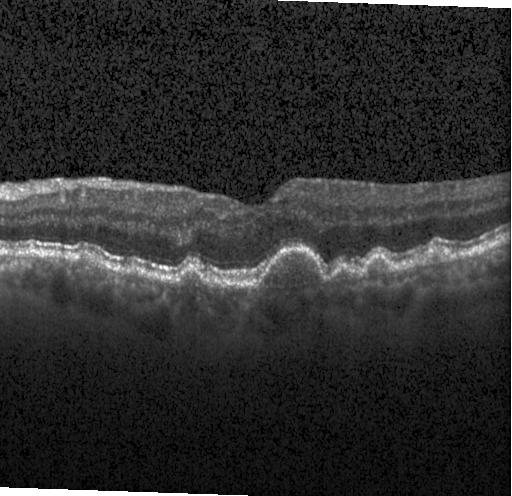 OCT finding: multiple drusen.